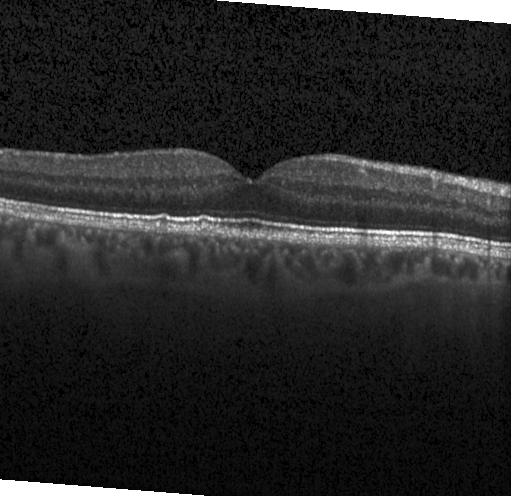
Finding: sub-RPE drusenoid deposits.